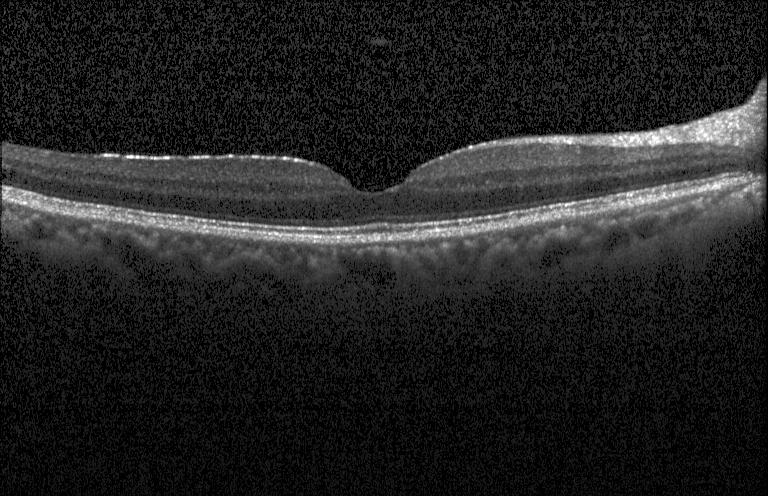
OCT line scan, instrument: Heidelberg Spectralis, through the macula
Dx: no choroidal neovascularization, diabetic macular edema, or drusen.